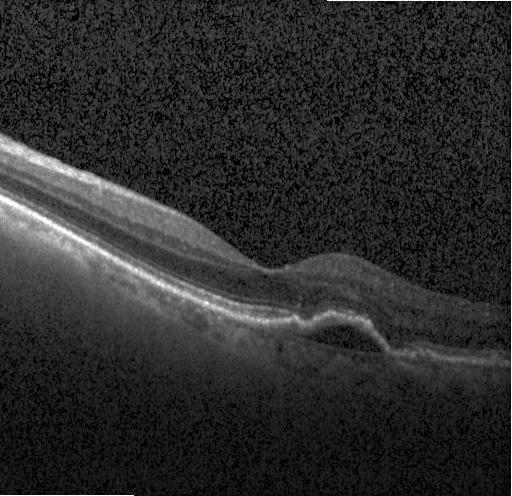
Horizontal scan through the fovea; SD-OCT; OCT B-scan; acquired on a Heidelberg Spectralis.
This B-scan demonstrates choroidal neovascularization.